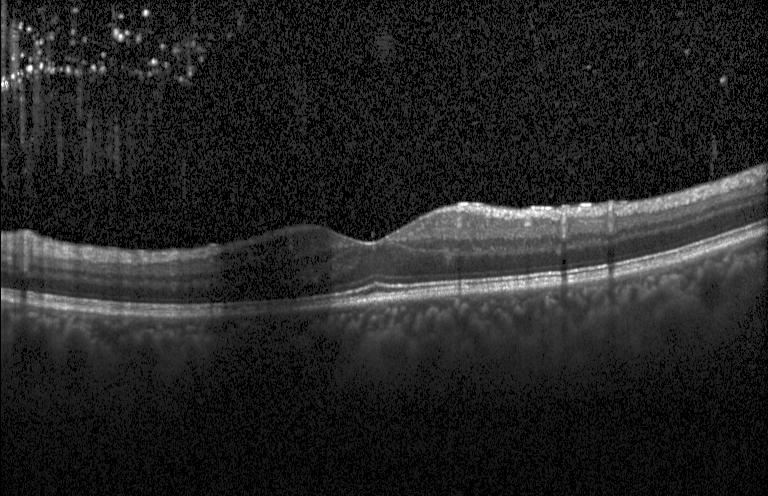
Heidelberg Spectralis, fovea-centered, retinal OCT B-scan, spectral-domain optical coherence tomography
Diagnosis: no choroidal neovascularization, no diabetic macular edema, and no drusen.